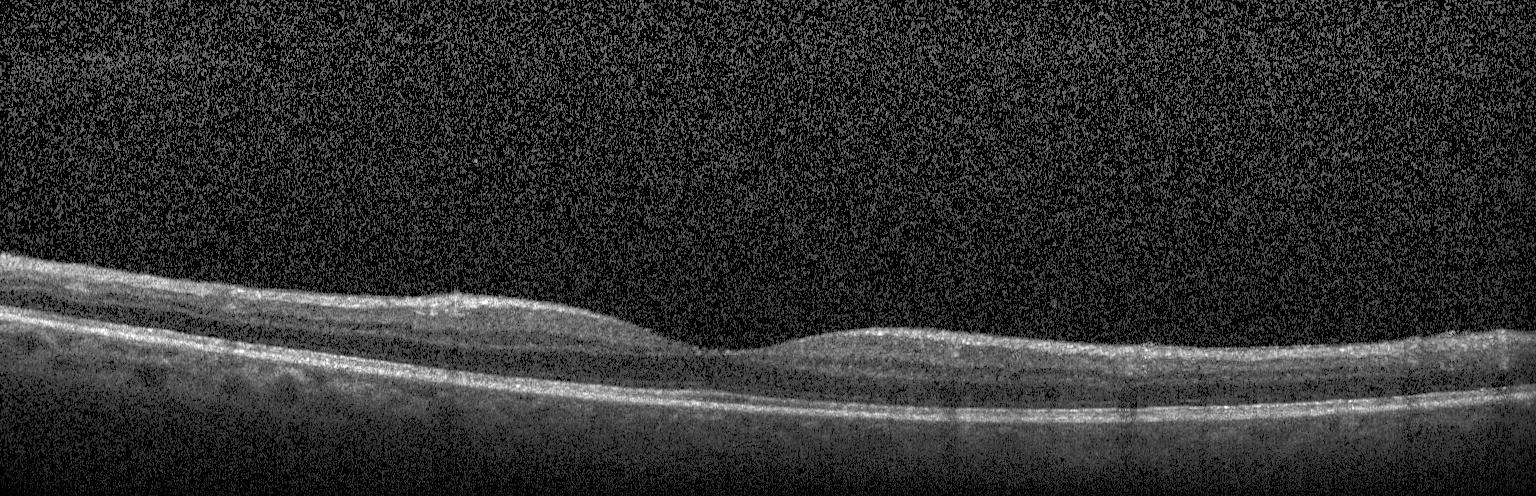

Macular OCT: no CNV, DME, or drusen.